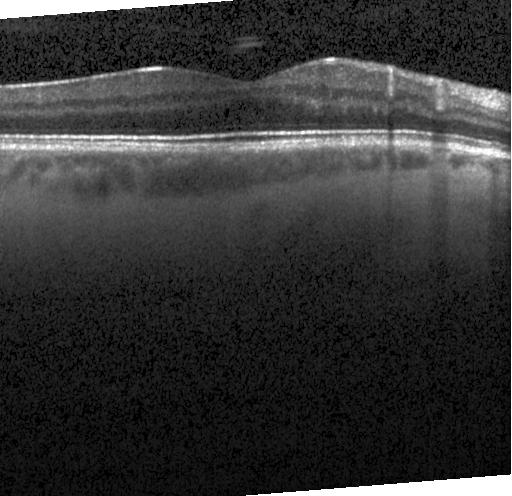 Retinal OCT B-scan
Assessment: no evidence of choroidal neovascularization, diabetic macular edema, or drusen.